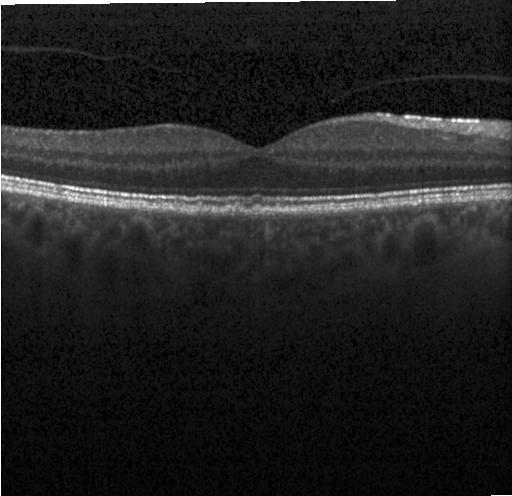
Impression: multiple drusen.